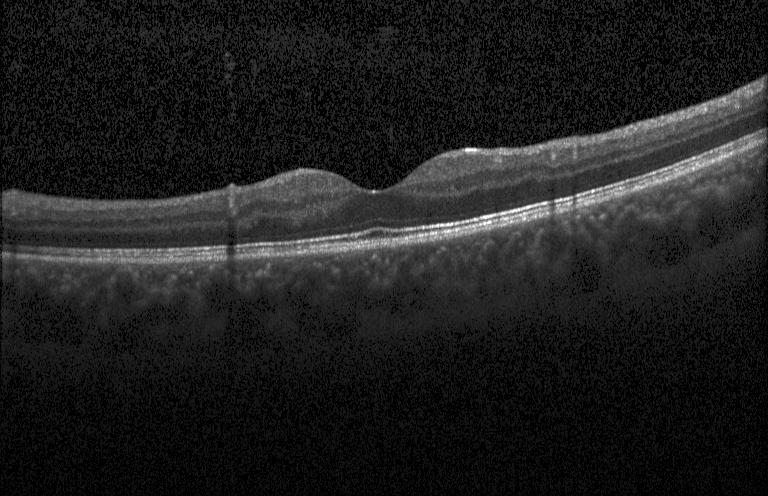 Optical coherence tomography scan. Heidelberg Spectralis OCT system. Diagnosis: no choroidal neovascularization, diabetic macular edema, or drusen.